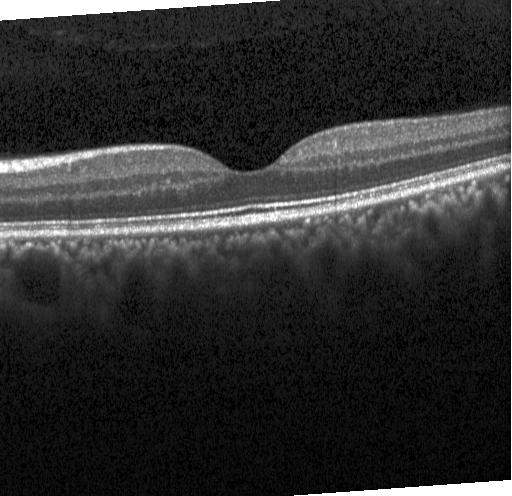 Macular OCT demonstrating no choroidal neovascularization, no diabetic macular edema, and no drusen.